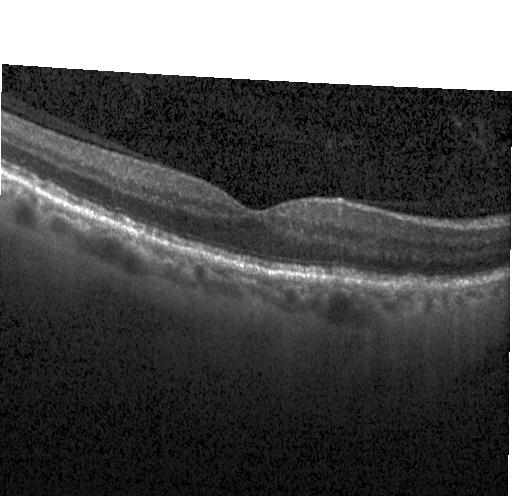

Retinal OCT B-scan, Heidelberg Spectralis, macular scan
Diagnosis: no evidence of choroidal neovascularization, diabetic macular edema, or drusen.